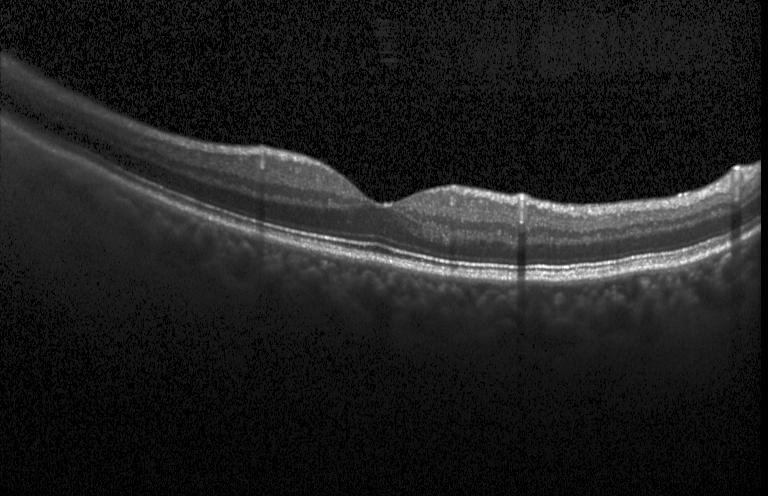 Diagnosis: no CNV, DME, or drusen.